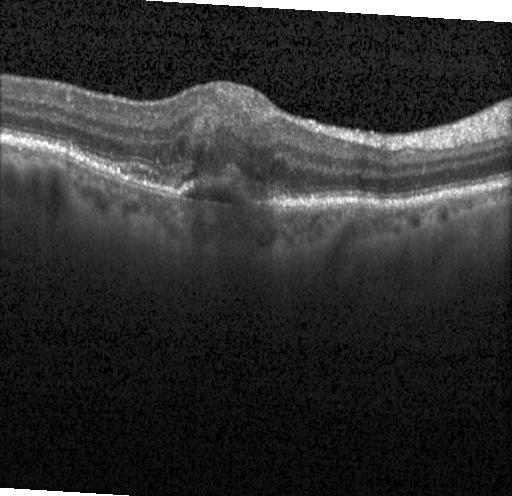
Through the macula; OCT line scan; instrument: Heidelberg Spectralis; spectral-domain optical coherence tomography
Assessment: choroidal neovascularization (CNV).